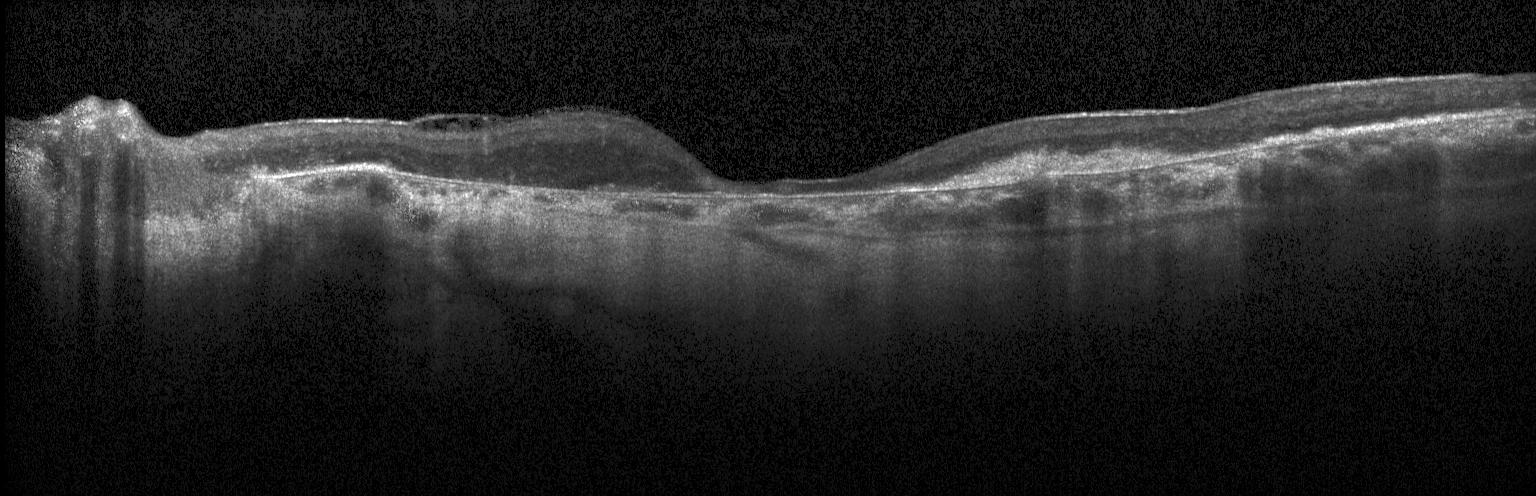

Retinal OCT B-scan
Choroidal neovascularization.